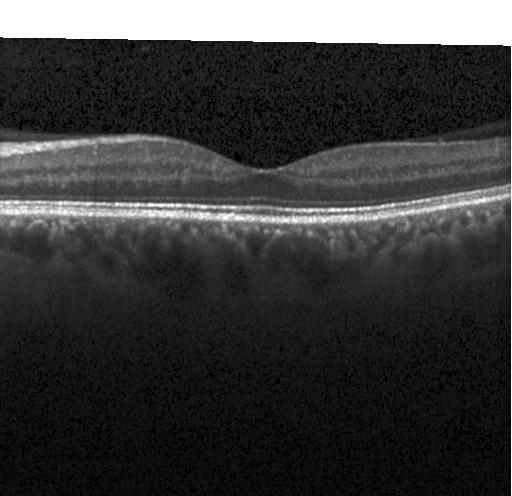

Fovea-centered · Heidelberg Spectralis · SD-OCT · retinal OCT B-scan. Finding: no CNV, DME, or drusen.